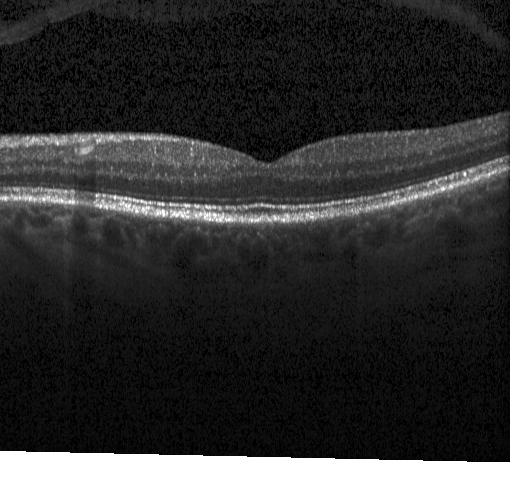

Retinal OCT B-scan.
Assessment: no choroidal neovascularization, no diabetic macular edema, and no drusen.